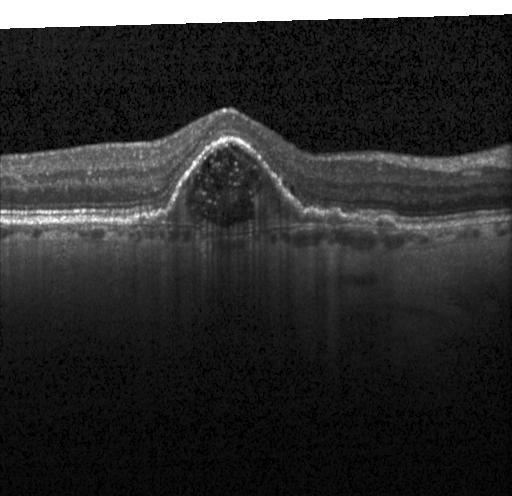
Macular OCT: a choroidal neovascular membrane.